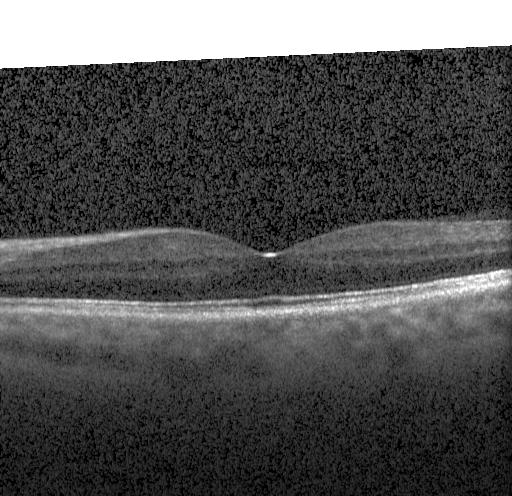
OCT line scan — This B-scan demonstrates neither choroidal neovascularization, diabetic macular edema, nor drusen.